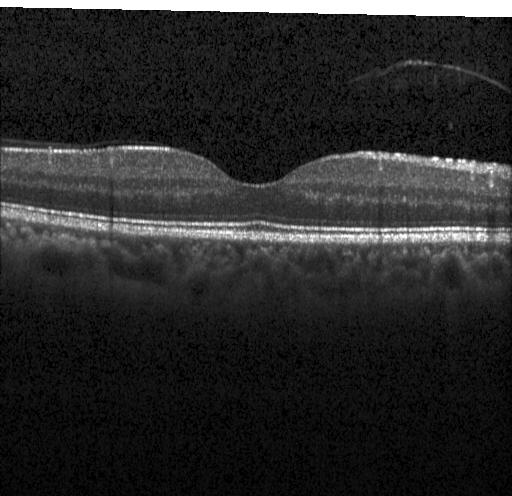
Heidelberg Spectralis OCT system; spectral-domain optical coherence tomography; optical coherence tomography scan. This B-scan demonstrates no choroidal neovascularization, diabetic macular edema, or drusen.